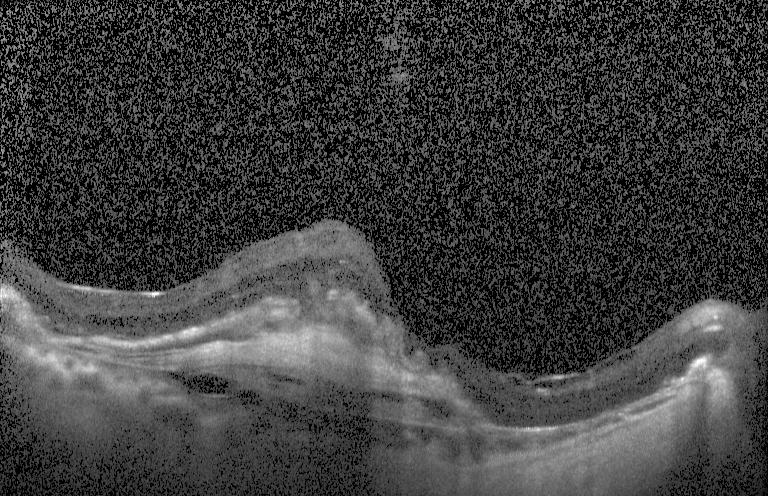
Impression: a choroidal neovascular membrane.